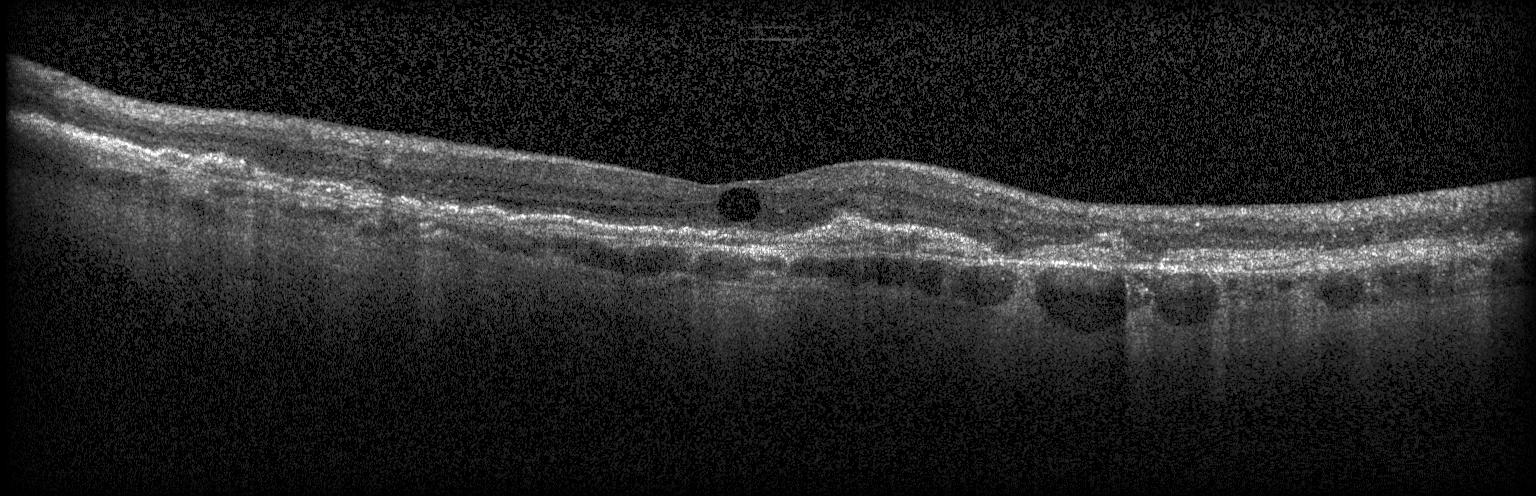

Impression: choroidal neovascularization.